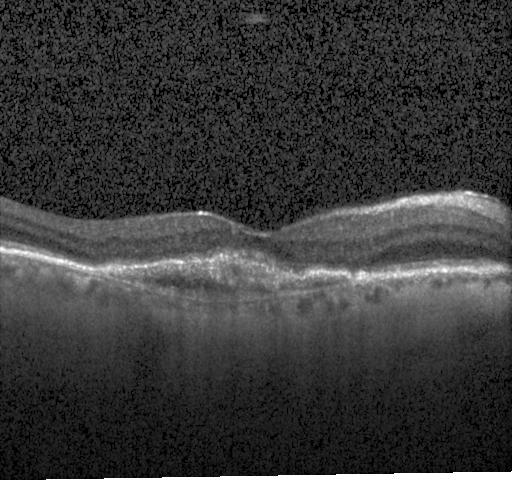
Instrument: Heidelberg Spectralis. OCT line scan. Macular scan.
The scan shows CNV.